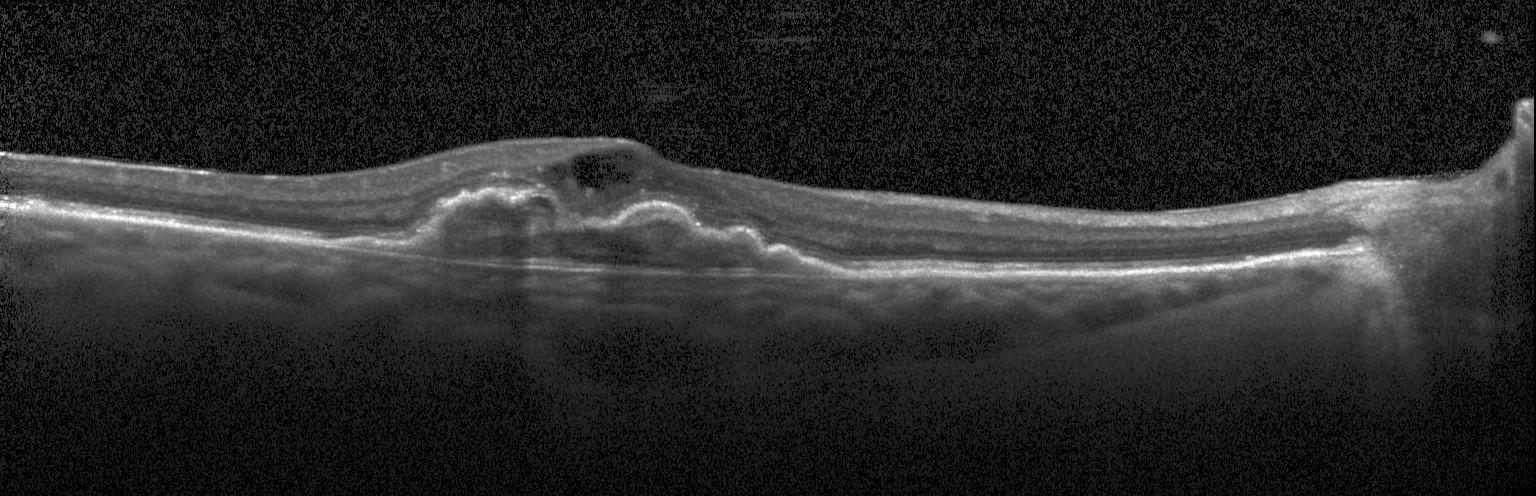 Macular OCT: a choroidal neovascular membrane.